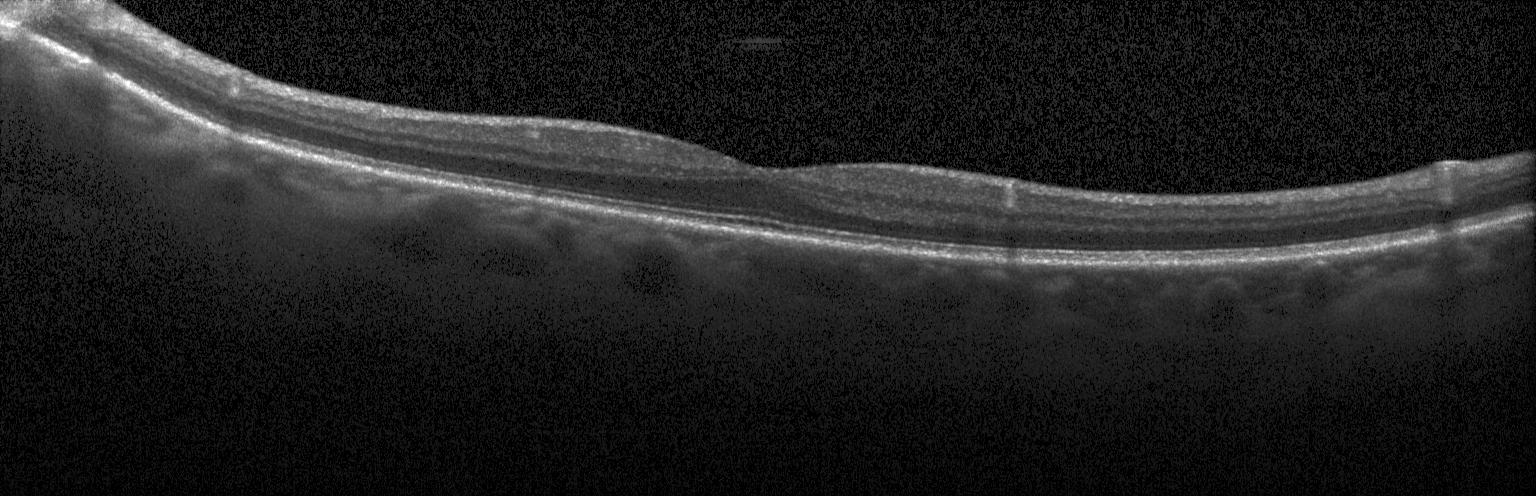 Optical coherence tomography scan; spectral-domain optical coherence tomography; horizontal scan through the fovea. The scan shows neither CNV, DME, nor drusen.